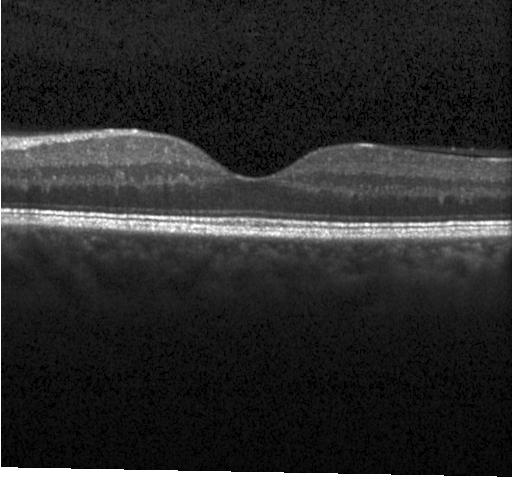

Through the macula; OCT line scan.
Diagnosis: no choroidal neovascularization, no diabetic macular edema, and no drusen.